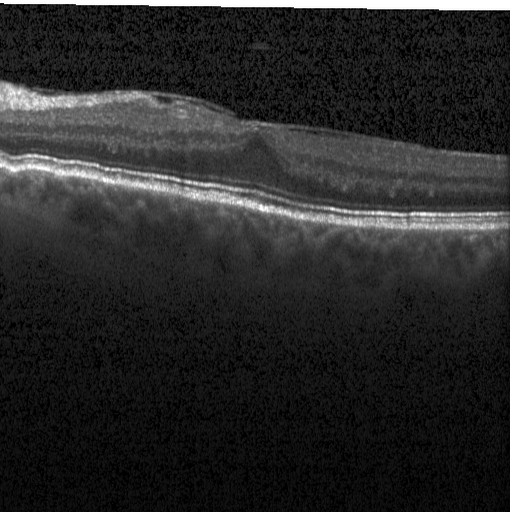
OCT line scan, horizontal scan through the fovea. Impression: diabetic macular edema (DME).